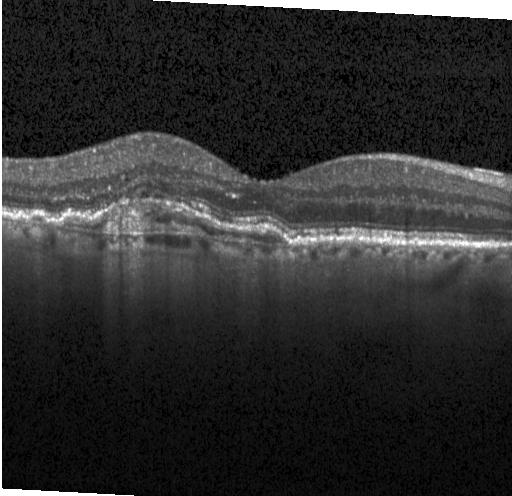

Retinal OCT cross-section.
Impression: a choroidal neovascular membrane.